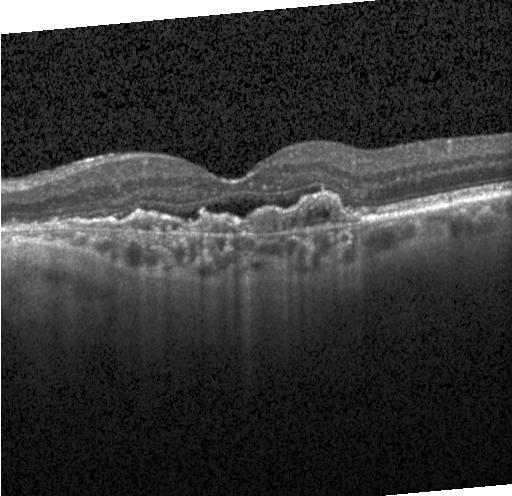
Macular OCT demonstrating choroidal neovascularization.